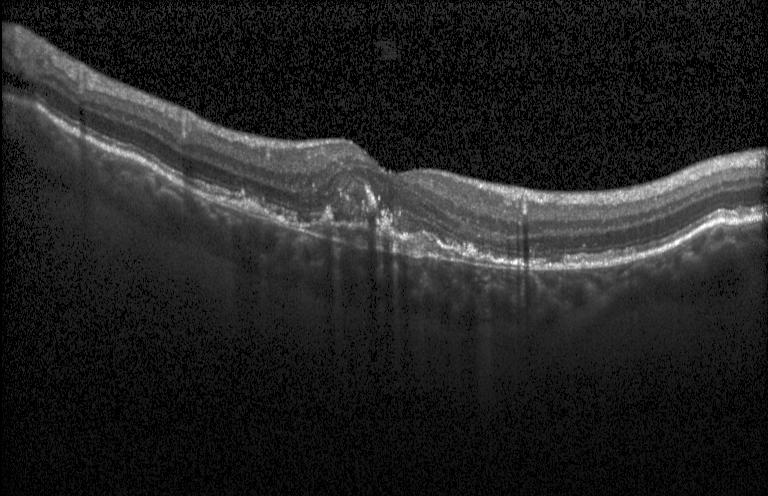 CNV.